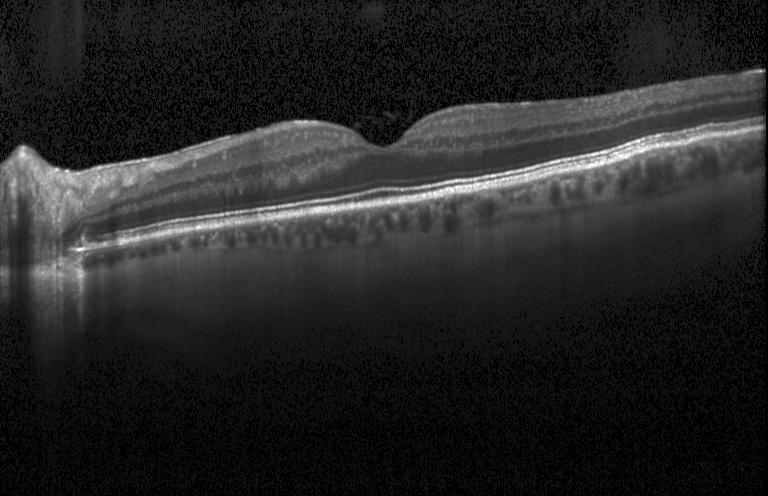
Retinal OCT cross-section, spectral-domain optical coherence tomography, macular scan, acquired on a Heidelberg Spectralis — Neither choroidal neovascularization, diabetic macular edema, nor drusen.